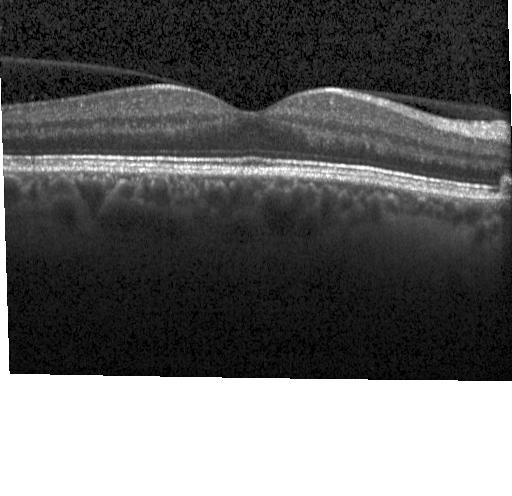 Impression: drusen.